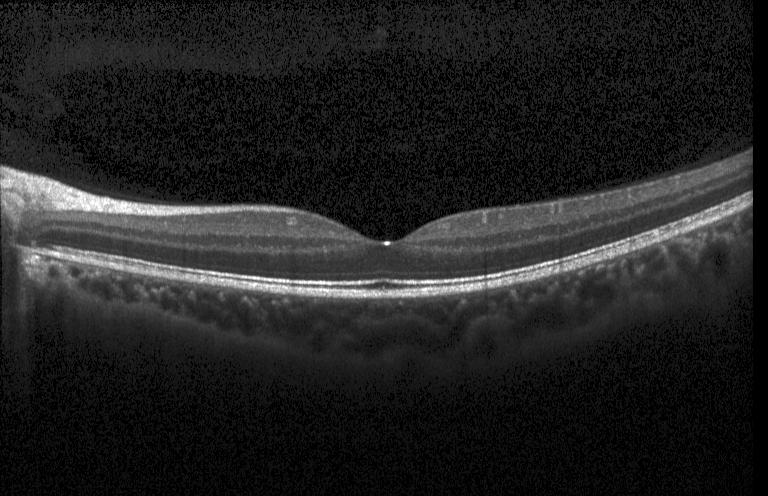 Retinal OCT cross-section showing no CNV, no DME, and no drusen.